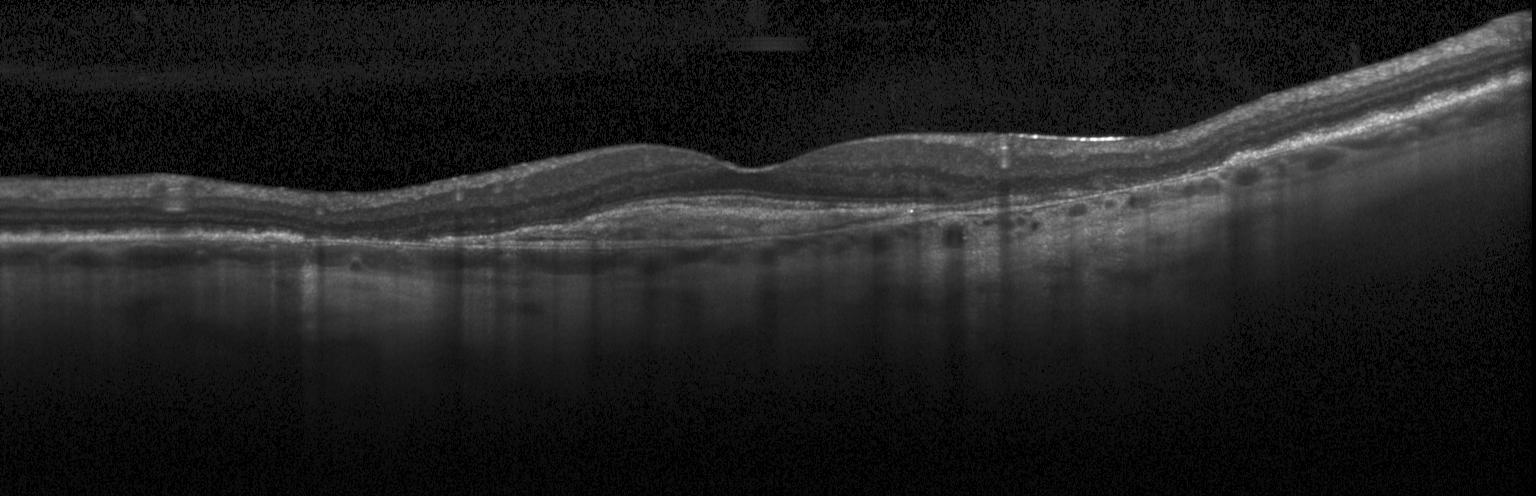 This B-scan demonstrates a choroidal neovascular membrane.